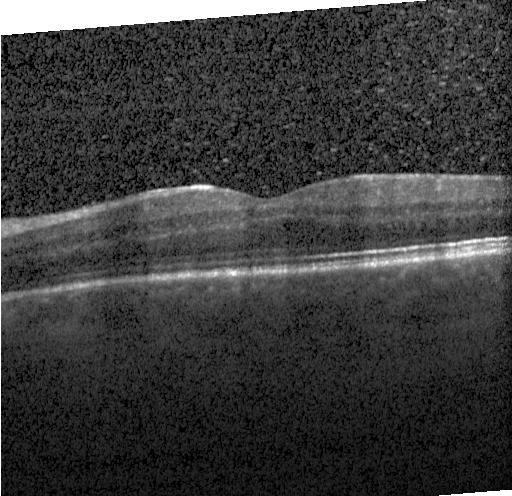
Optical coherence tomography B-scan — Diagnosis: neither choroidal neovascularization, diabetic macular edema, nor drusen.